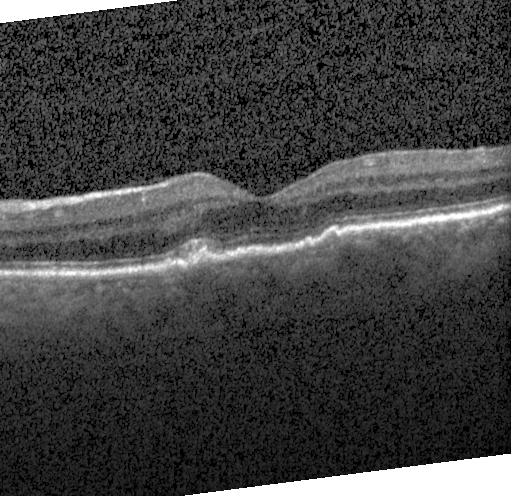

The scan shows sub-RPE drusenoid deposits.